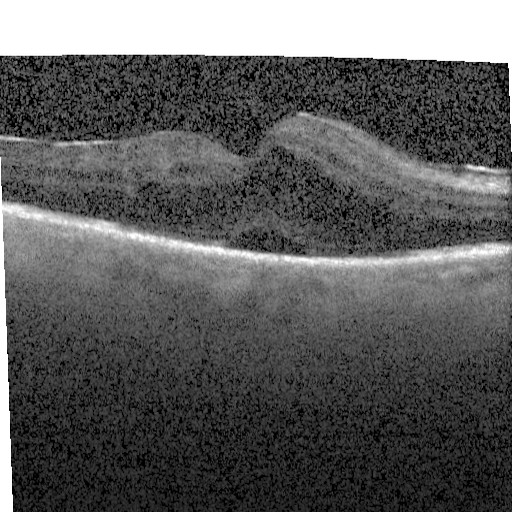

Spectral-domain OCT B-scan: diabetic macular edema (DME).